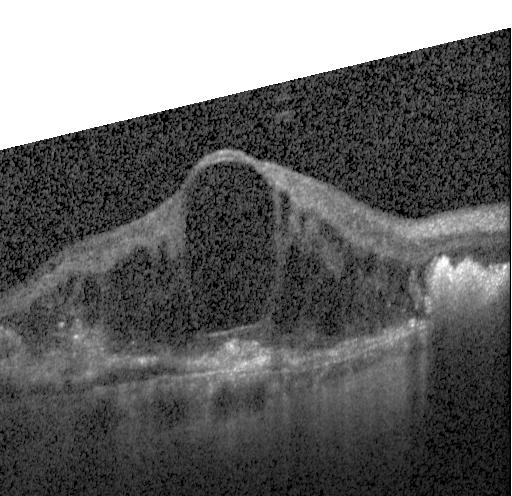

SD-OCT; OCT B-scan; centered on the fovea; Heidelberg Spectralis — Finding: CNV.